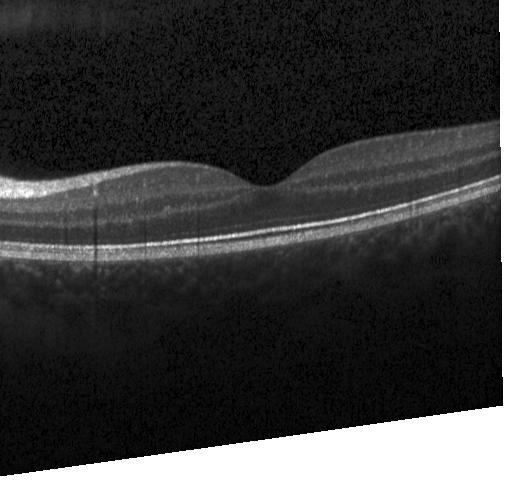
Finding: neither choroidal neovascularization, diabetic macular edema, nor drusen.